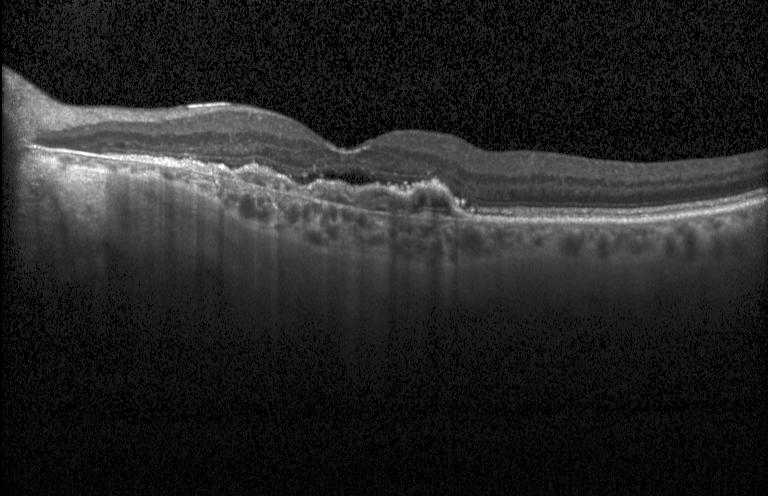 Fovea-centered. Heidelberg Spectralis OCT system. SD-OCT. OCT line scan
Finding: choroidal neovascularization.